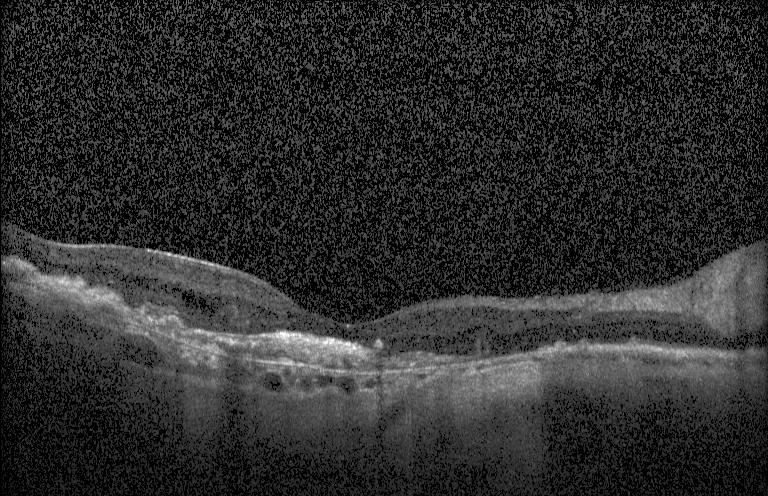
OCT B-scan showing CNV.